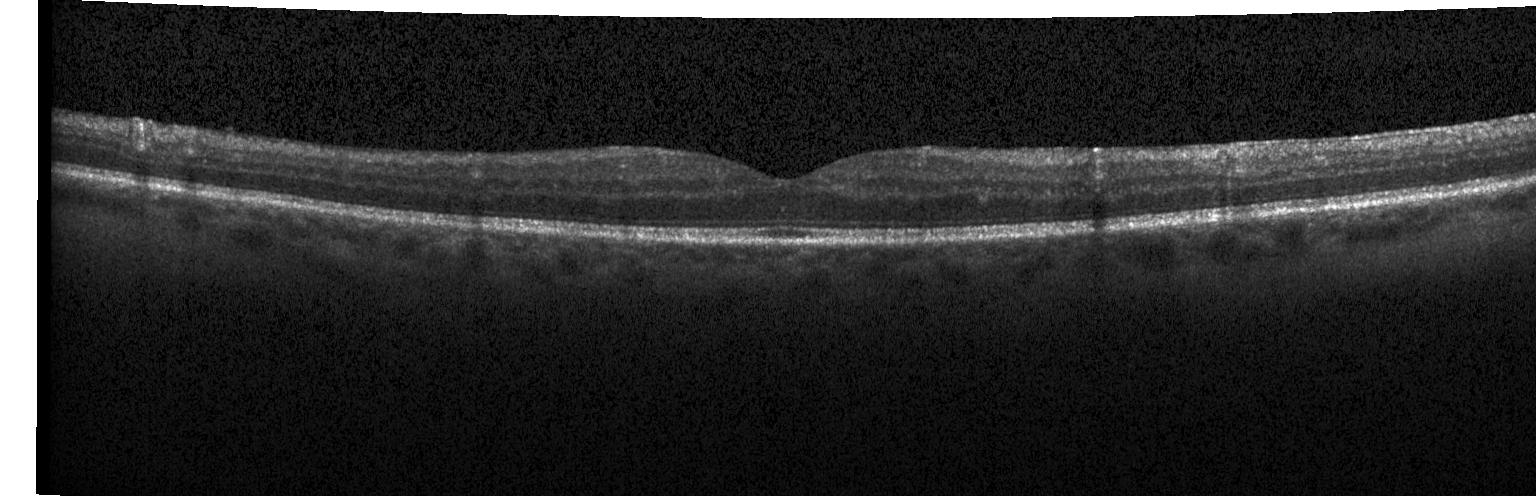

Macular OCT: no evidence of CNV, DME, or drusen.